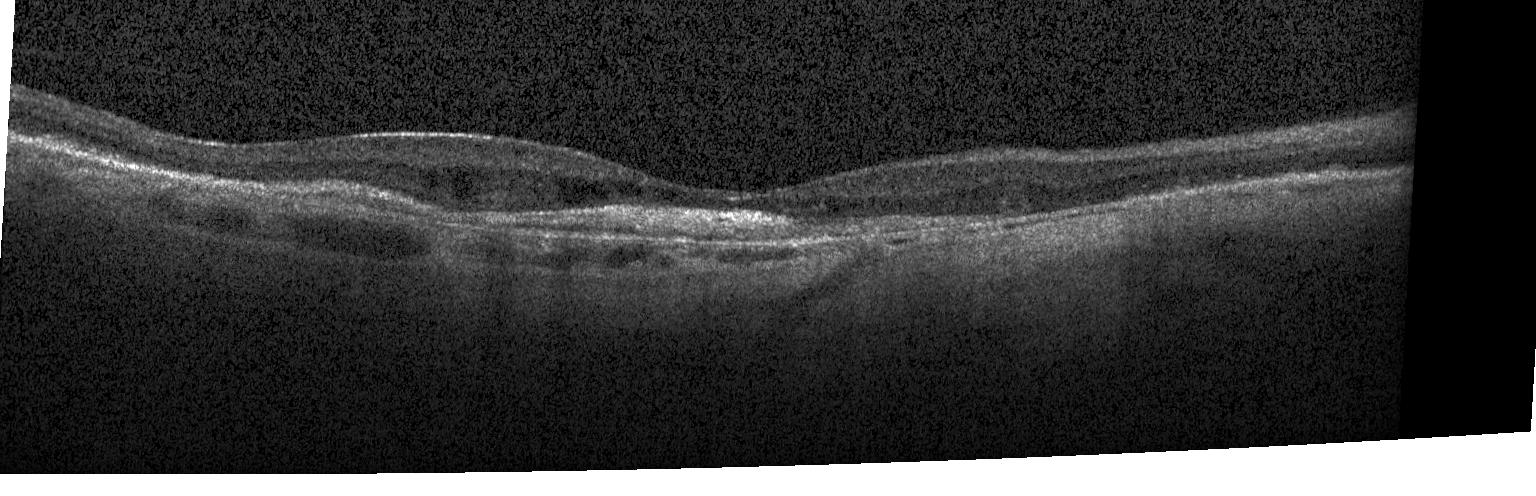 Horizontal scan through the fovea. SD-OCT. OCT line scan.
Choroidal neovascularization.